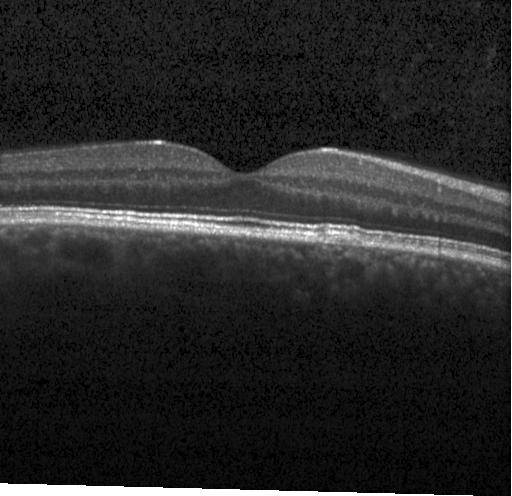
Finding: no CNV, DME, or drusen.